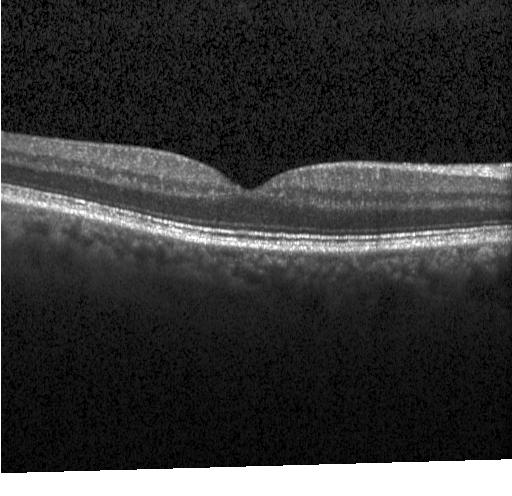
Finding: no evidence of CNV, DME, or drusen.